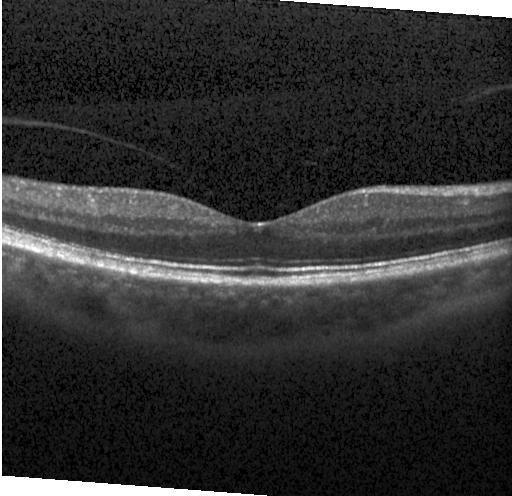

OCT line scan
The scan shows no evidence of choroidal neovascularization, diabetic macular edema, or drusen.